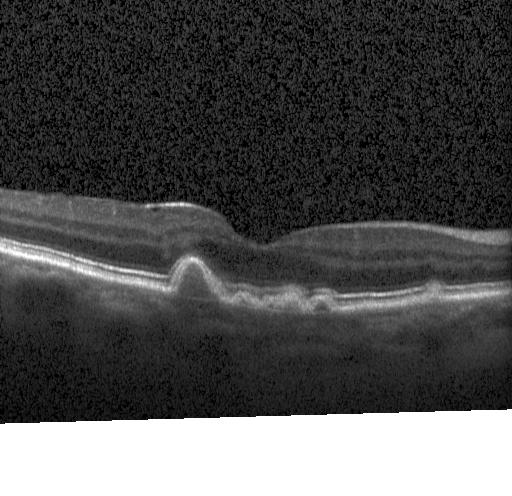
OCT B-scan; centered on the fovea; spectral-domain OCT.
Finding: drusen.